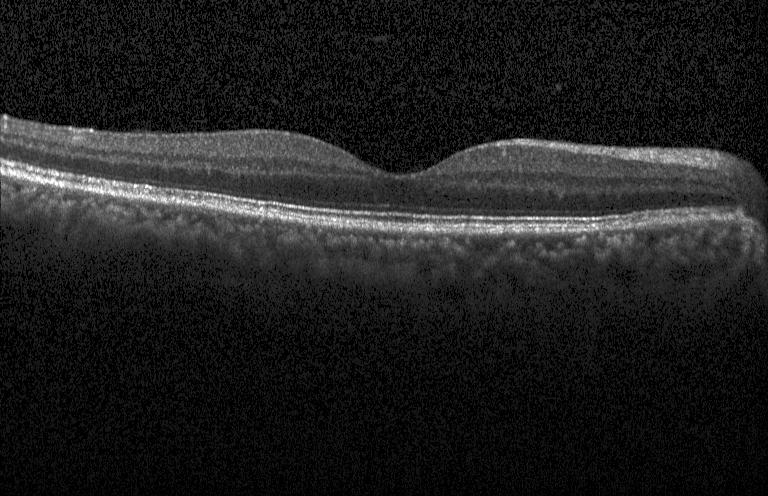 Impression: no choroidal neovascularization, no diabetic macular edema, and no drusen.